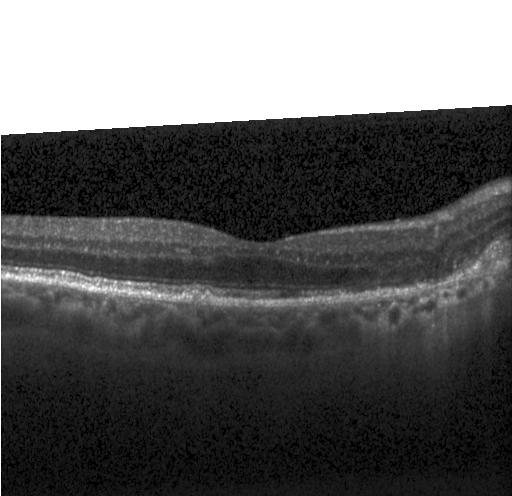

Impression: a choroidal neovascular membrane.